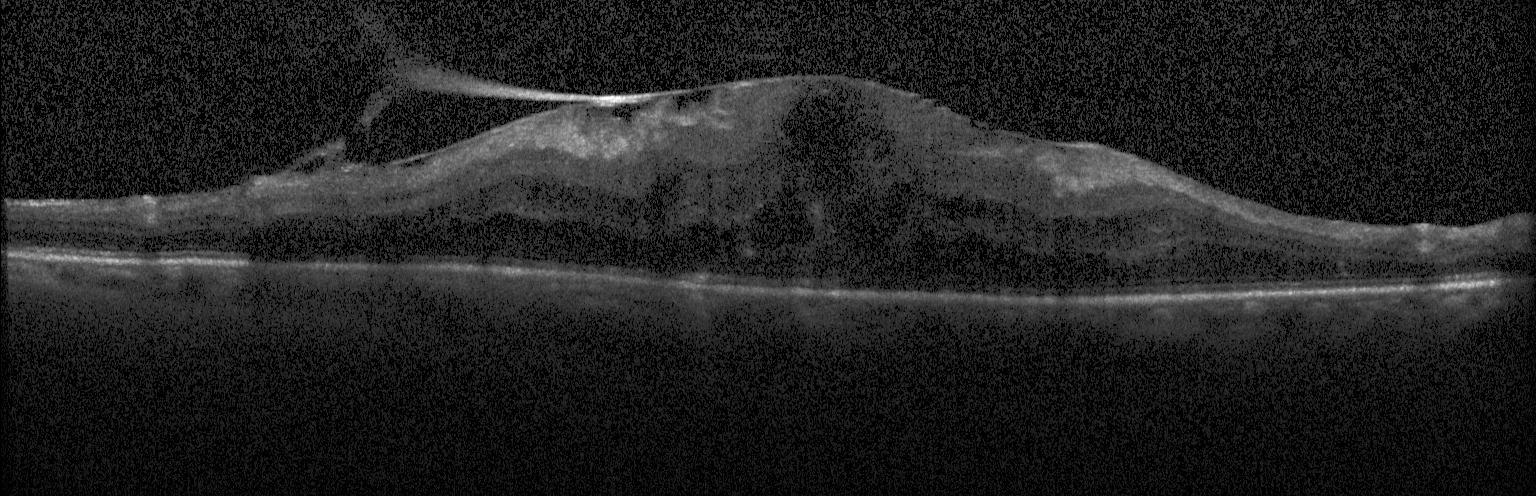

OCT B-scan, horizontal scan through the fovea, Heidelberg Spectralis OCT system, SD-OCT — Finding: diabetic macular edema.